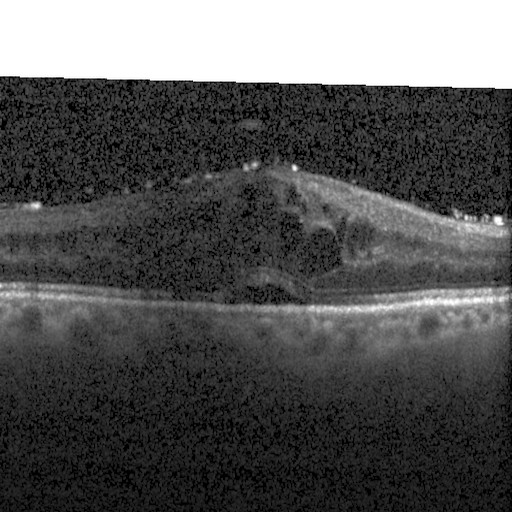
Through the macula; OCT B-scan. Diagnosis: DME.